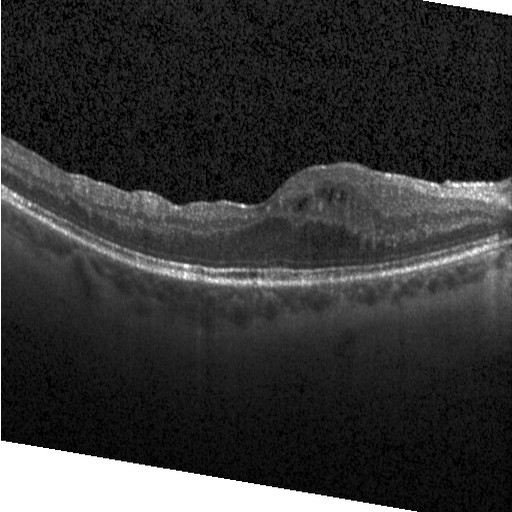
Spectral-domain OCT B-scan: diabetic macular edema.